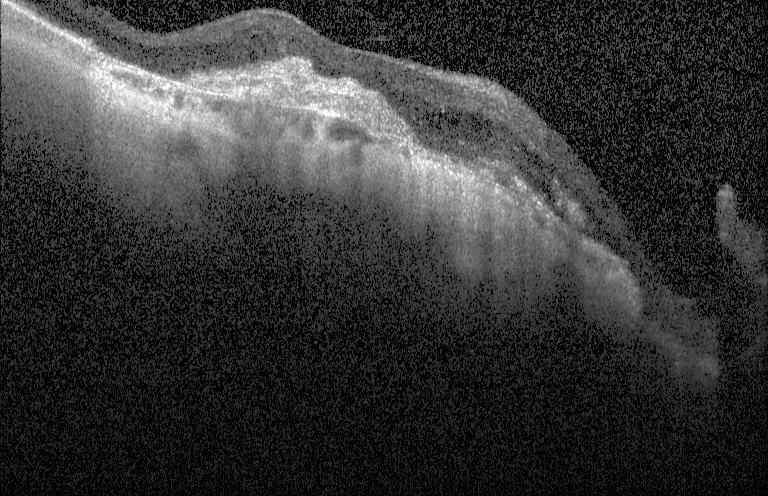
The scan shows a choroidal neovascular membrane.